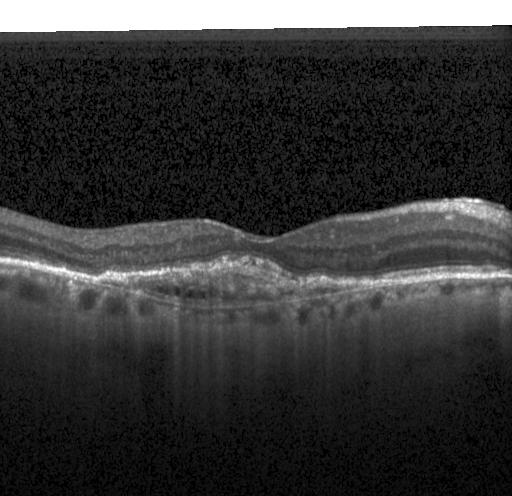
Macular OCT: a choroidal neovascular membrane.